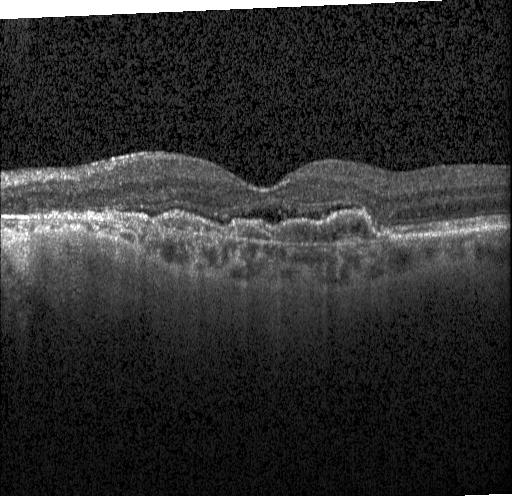
Optical coherence tomography B-scan.
Impression: CNV.